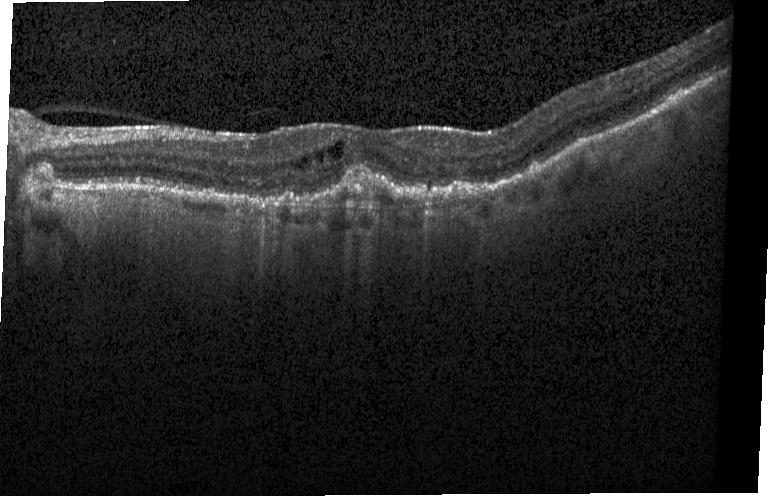

Impression: CNV.